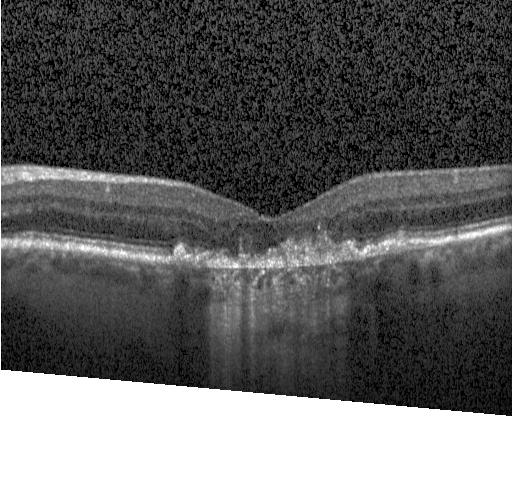

Optical coherence tomography scan.
The scan shows a choroidal neovascular membrane.